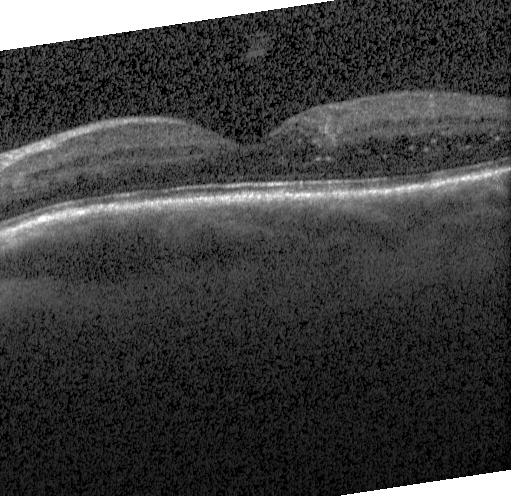
Retinal OCT cross-section.
Diagnosis: diabetic macular edema (DME).